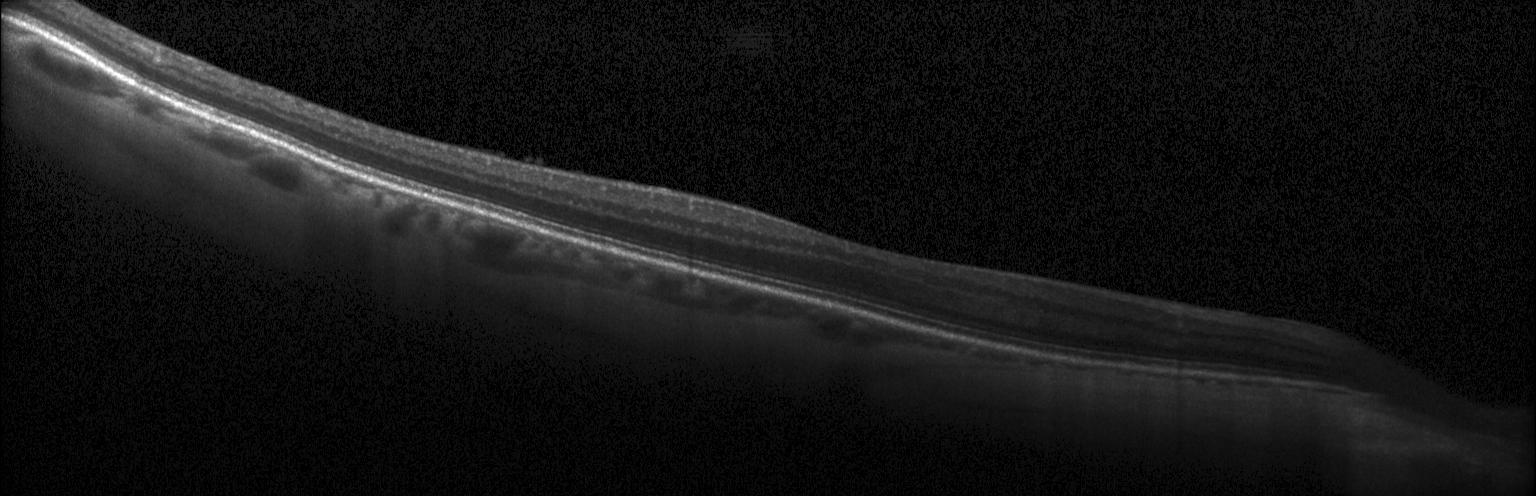

Retinal OCT B-scan. Macular scan.
Finding: no evidence of choroidal neovascularization, diabetic macular edema, or drusen.